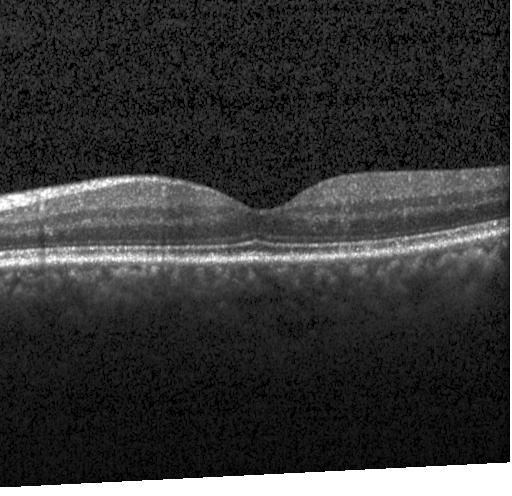

OCT finding: no CNV, no DME, and no drusen.